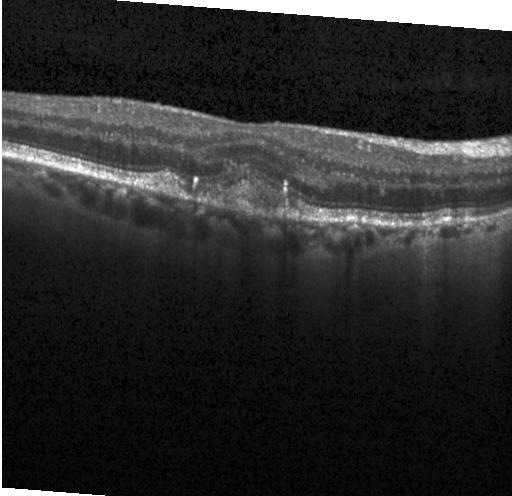

Assessment: a choroidal neovascular membrane.